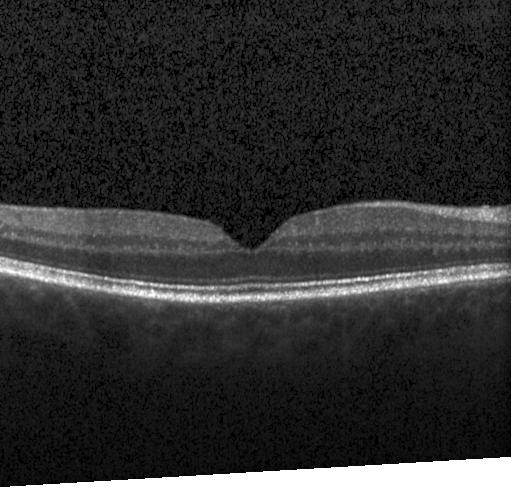

Retinal OCT cross-section
Assessment: no choroidal neovascularization, no diabetic macular edema, and no drusen.